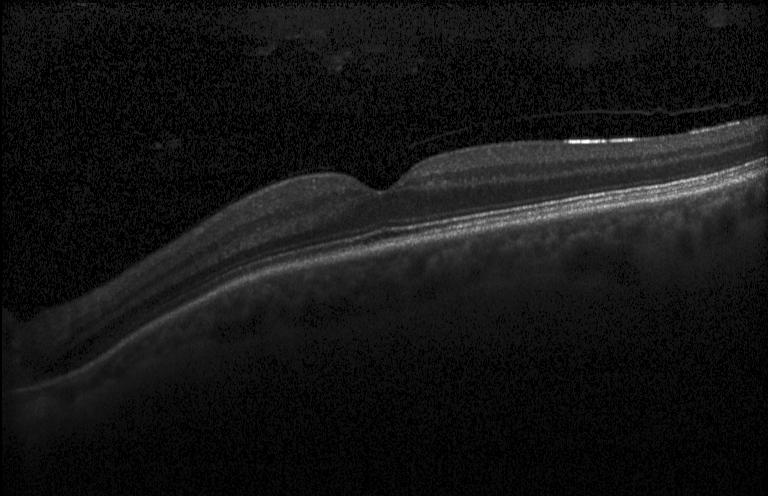 Spectral-domain optical coherence tomography · OCT line scan.
Dx: no evidence of choroidal neovascularization, diabetic macular edema, or drusen.